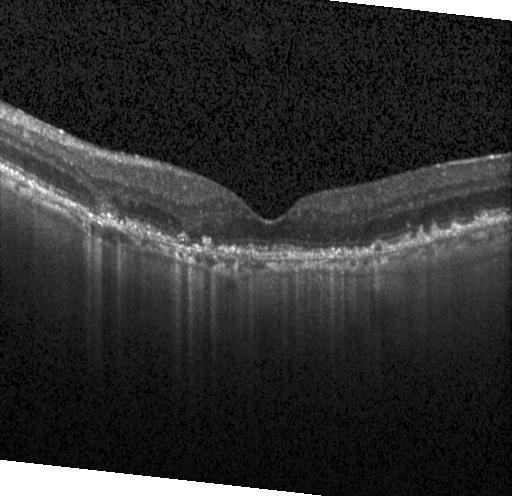 Spectral-domain OCT B-scan: a choroidal neovascular membrane.